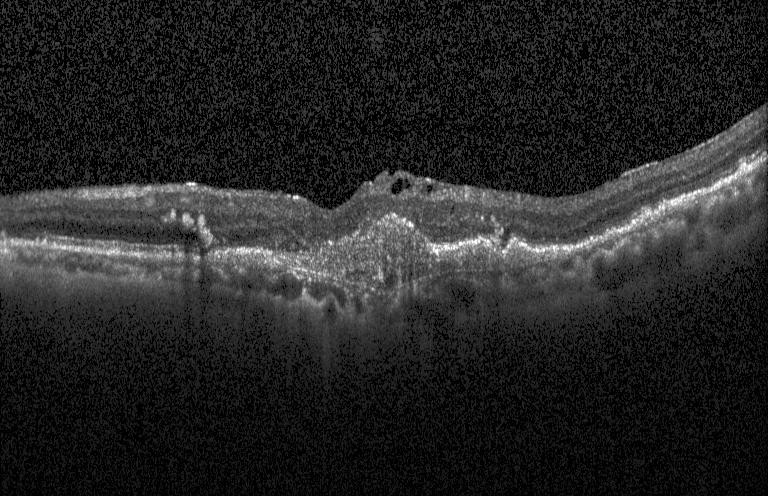

Impression: choroidal neovascularization.